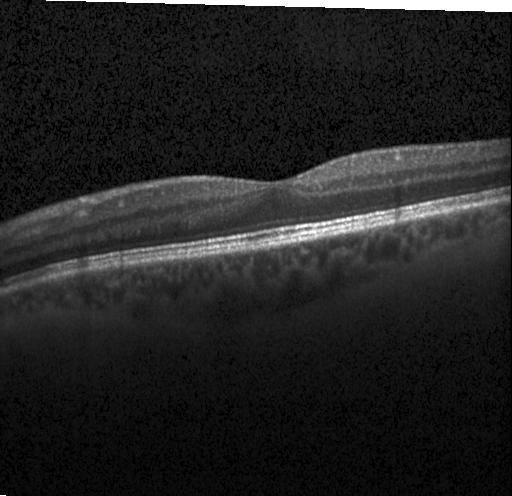

Dx: neither choroidal neovascularization, diabetic macular edema, nor drusen.